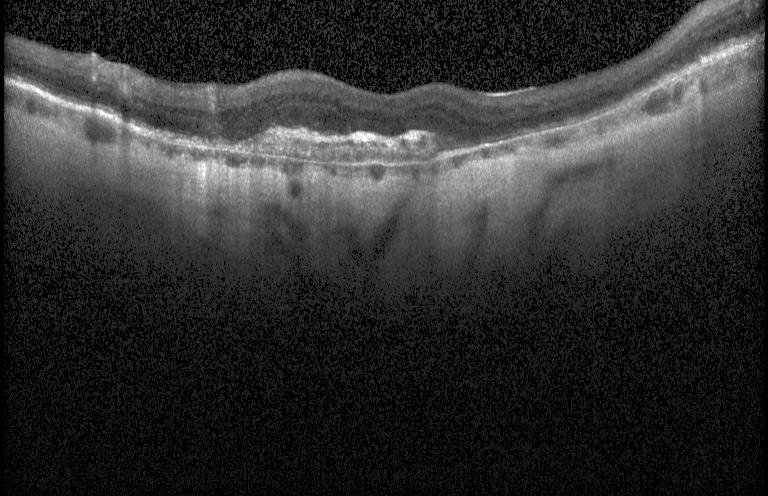

OCT line scan
Macular OCT: a choroidal neovascular membrane.